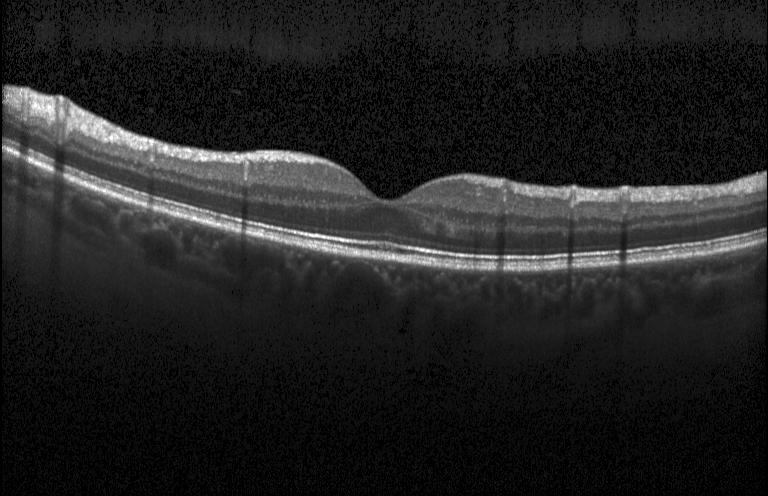 Macular OCT: neither choroidal neovascularization, diabetic macular edema, nor drusen.